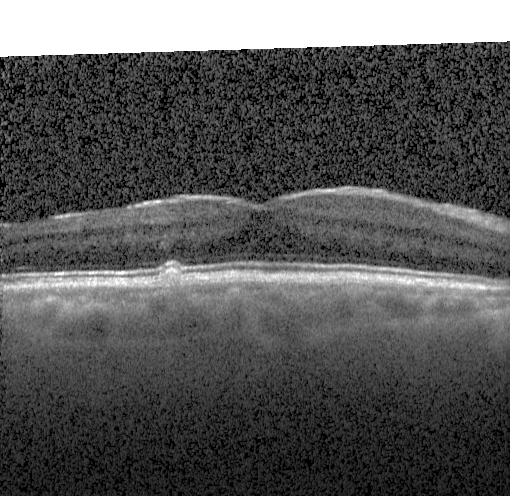 Spectral-domain OCT B-scan: drusen.